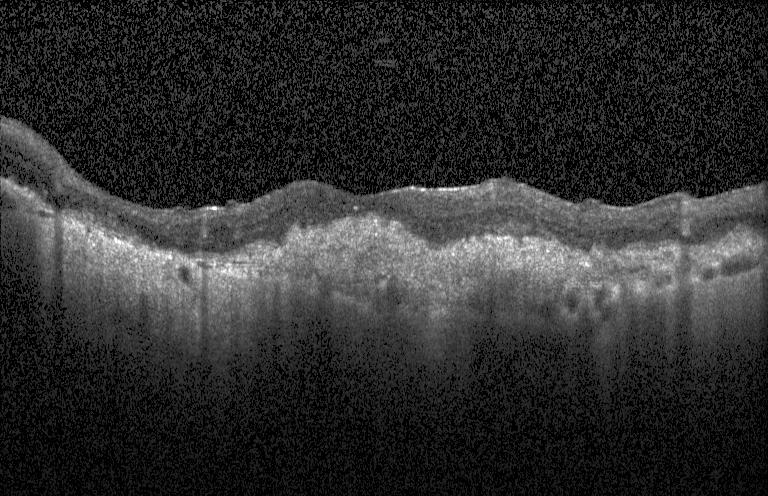
Acquired on a Heidelberg Spectralis, optical coherence tomography scan
Dx: choroidal neovascularization.